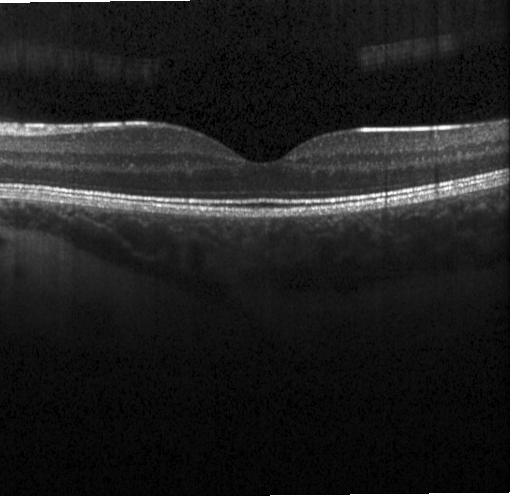

Through the macula. Heidelberg Spectralis. Optical coherence tomography scan.
Finding: neither CNV, DME, nor drusen.